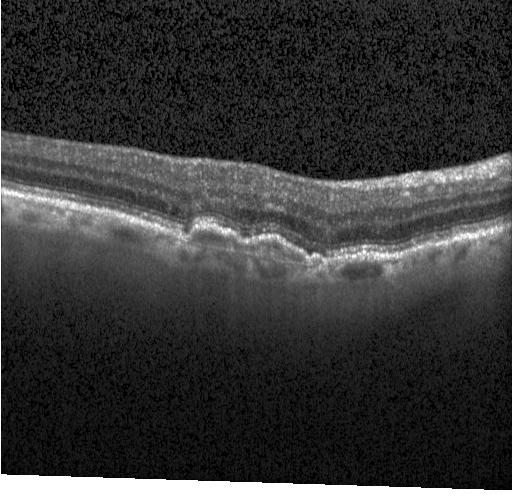
Retinal OCT B-scan, acquired on a Heidelberg Spectralis, spectral-domain optical coherence tomography, horizontal scan through the fovea. OCT finding: a choroidal neovascular membrane.